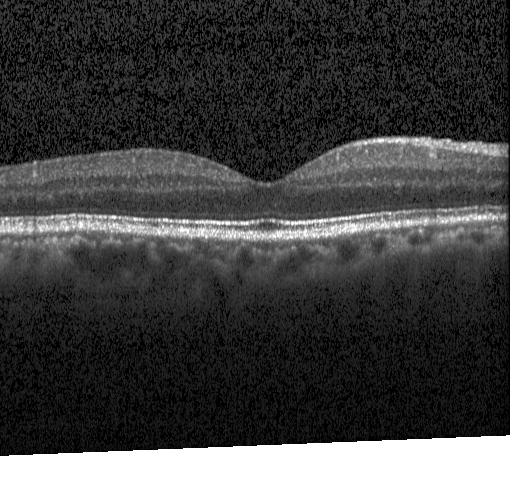

Diagnosis: no evidence of choroidal neovascularization, diabetic macular edema, or drusen.